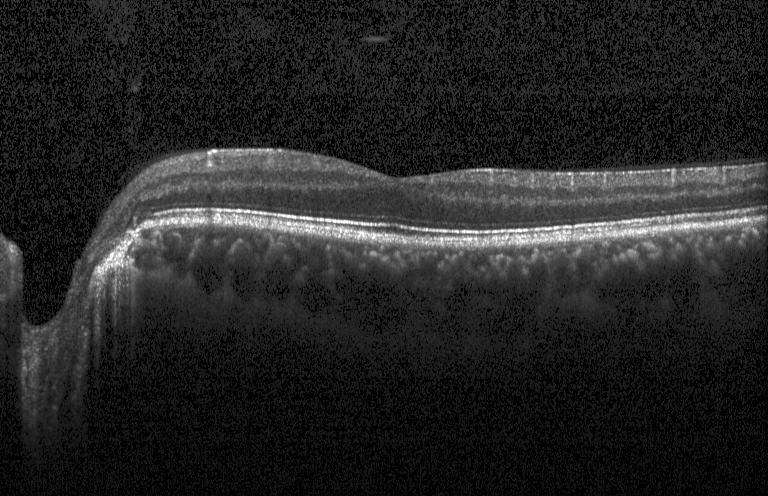
OCT B-scan showing no evidence of CNV, DME, or drusen.